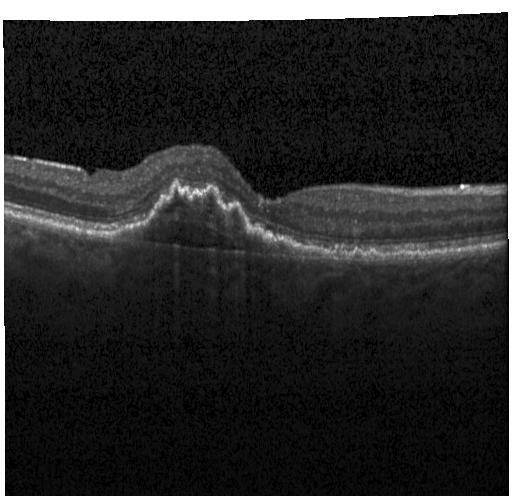
SD-OCT; optical coherence tomography B-scan; centered on the fovea — Macular OCT: choroidal neovascularization.